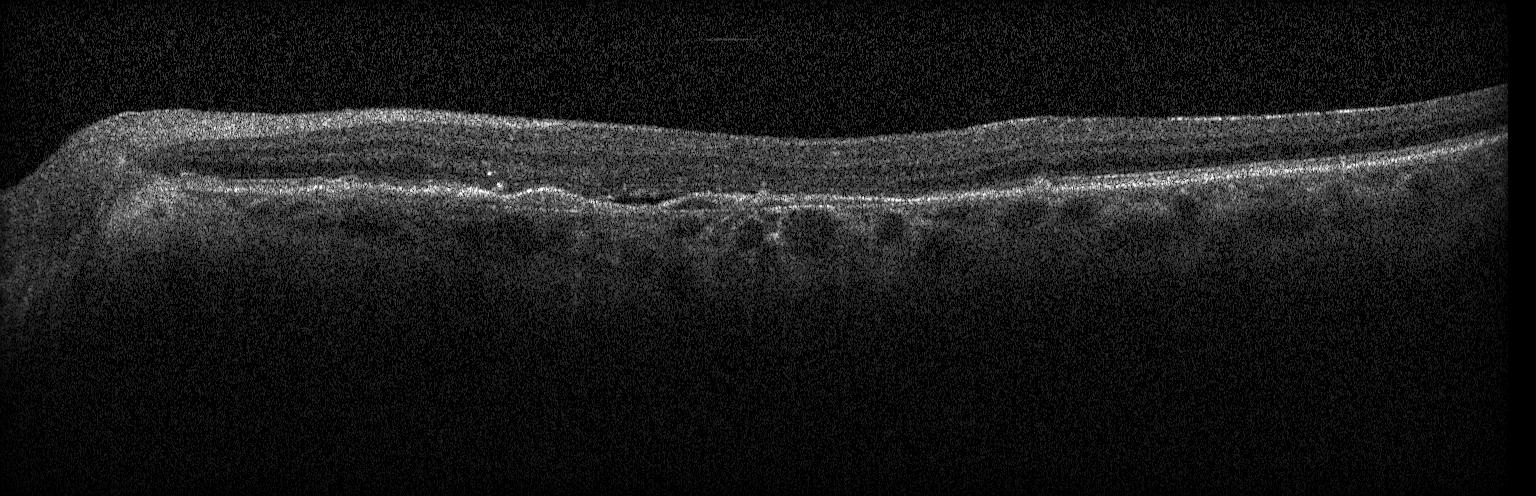

Finding: a choroidal neovascular membrane.